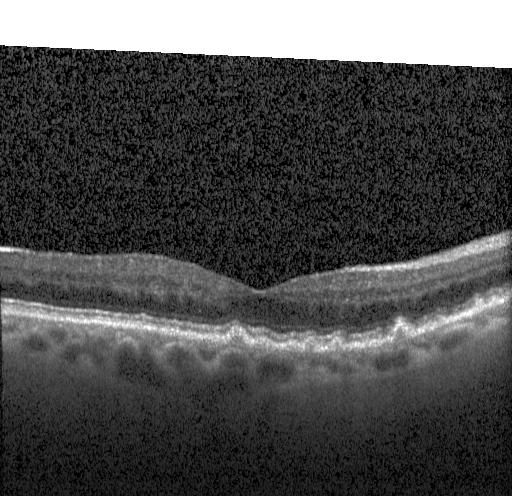 Optical coherence tomography B-scan · spectral-domain optical coherence tomography · acquired on a Heidelberg Spectralis · macular scan.
This B-scan demonstrates sub-RPE drusenoid deposits.